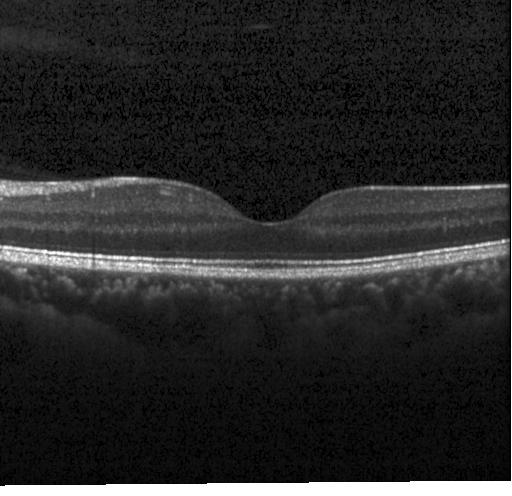
OCT line scan. Diagnosis: no evidence of choroidal neovascularization, diabetic macular edema, or drusen.